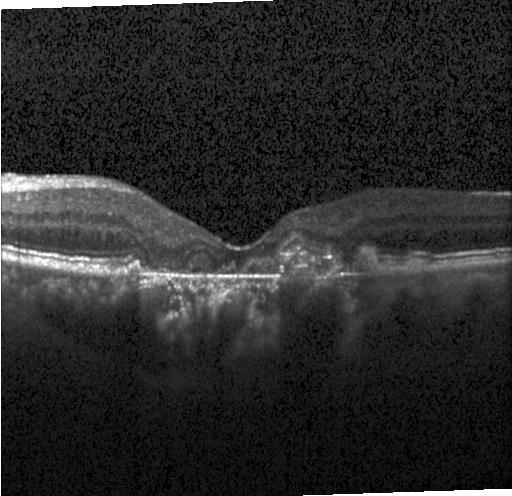
OCT scan showing a choroidal neovascular membrane.